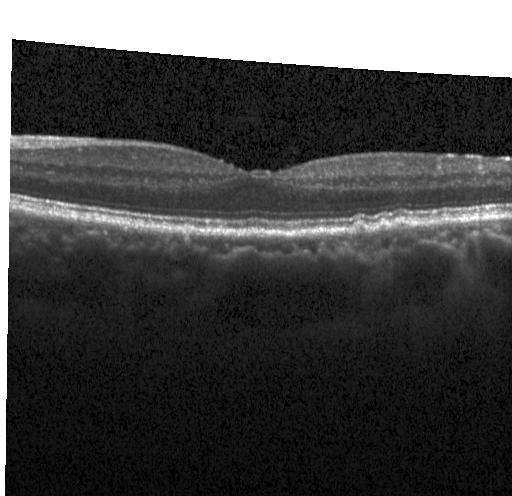

Macular scan; retinal OCT B-scan
Macular OCT: drusen.